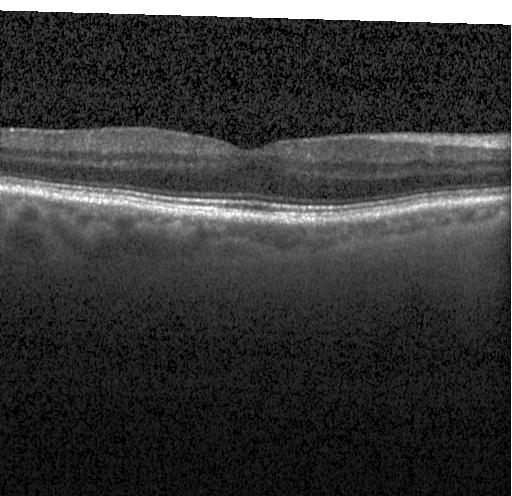 Spectral-domain optical coherence tomography. Optical coherence tomography scan. Macular scan
Neither choroidal neovascularization, diabetic macular edema, nor drusen.